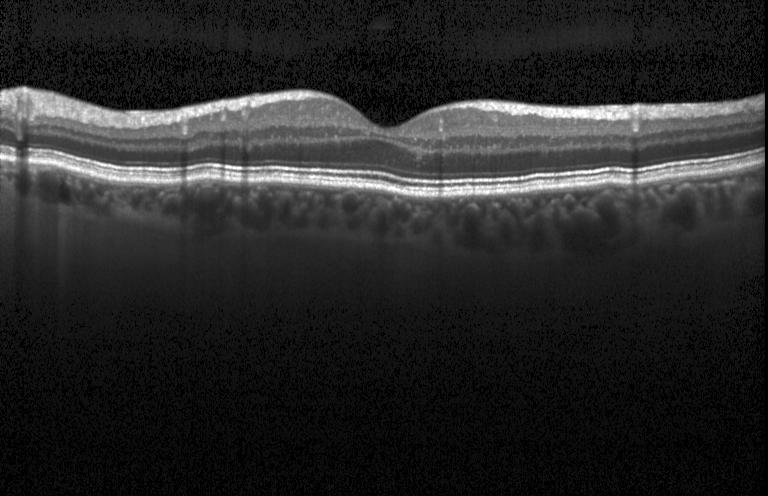
Retinal OCT cross-section, spectral-domain optical coherence tomography. Impression: no choroidal neovascularization, diabetic macular edema, or drusen.